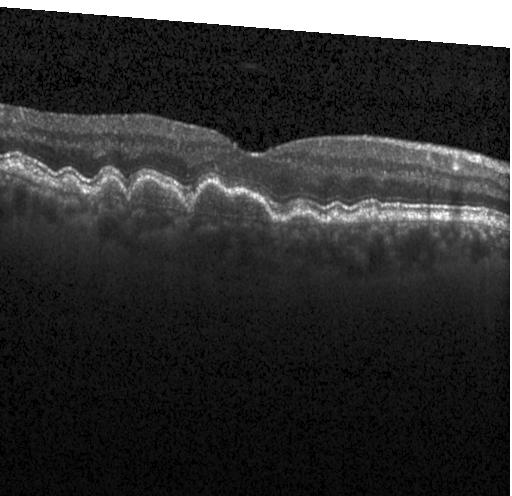

Macular OCT: multiple drusen.